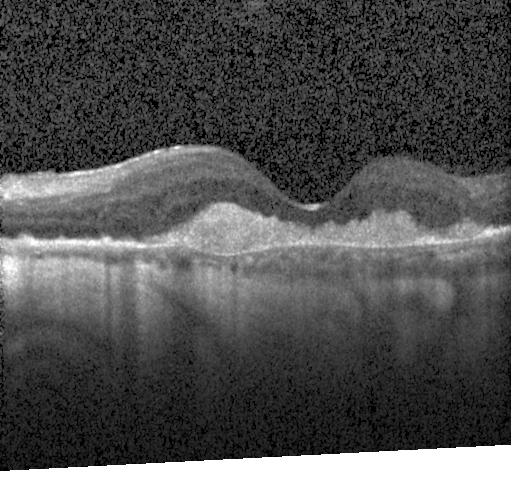 Macular OCT demonstrating a choroidal neovascular membrane.